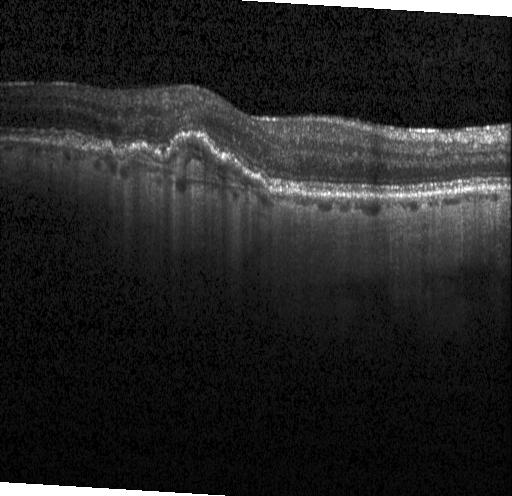 OCT line scan, spectral-domain OCT, acquired on a Heidelberg Spectralis — Diagnosis: CNV.